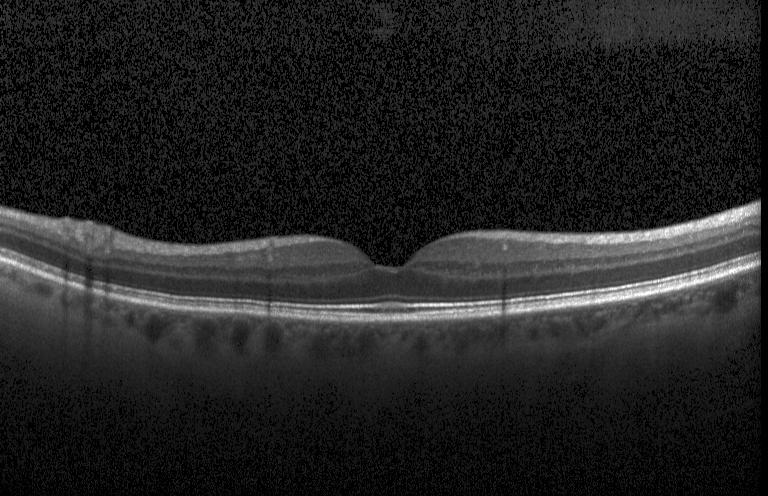
Optical coherence tomography B-scan; SD-OCT; through the macula; Heidelberg Spectralis OCT system
Impression: no choroidal neovascularization, diabetic macular edema, or drusen.